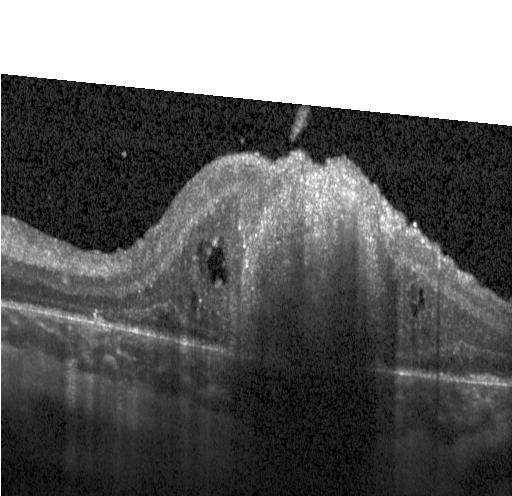
Horizontal scan through the fovea. Retinal OCT cross-section.
A choroidal neovascular membrane.